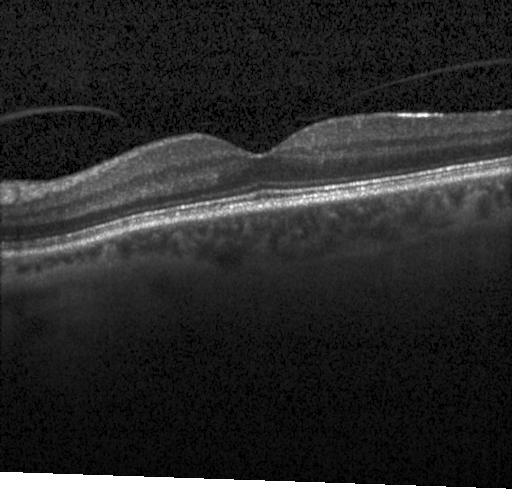
Retinal OCT B-scan — Diagnosis: no choroidal neovascularization, no diabetic macular edema, and no drusen.